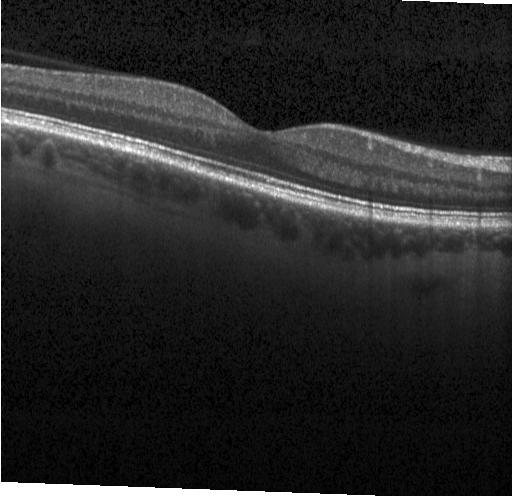 Retinal OCT B-scan; through the macula; SD-OCT; acquired on a Heidelberg Spectralis
Impression: no evidence of choroidal neovascularization, diabetic macular edema, or drusen.